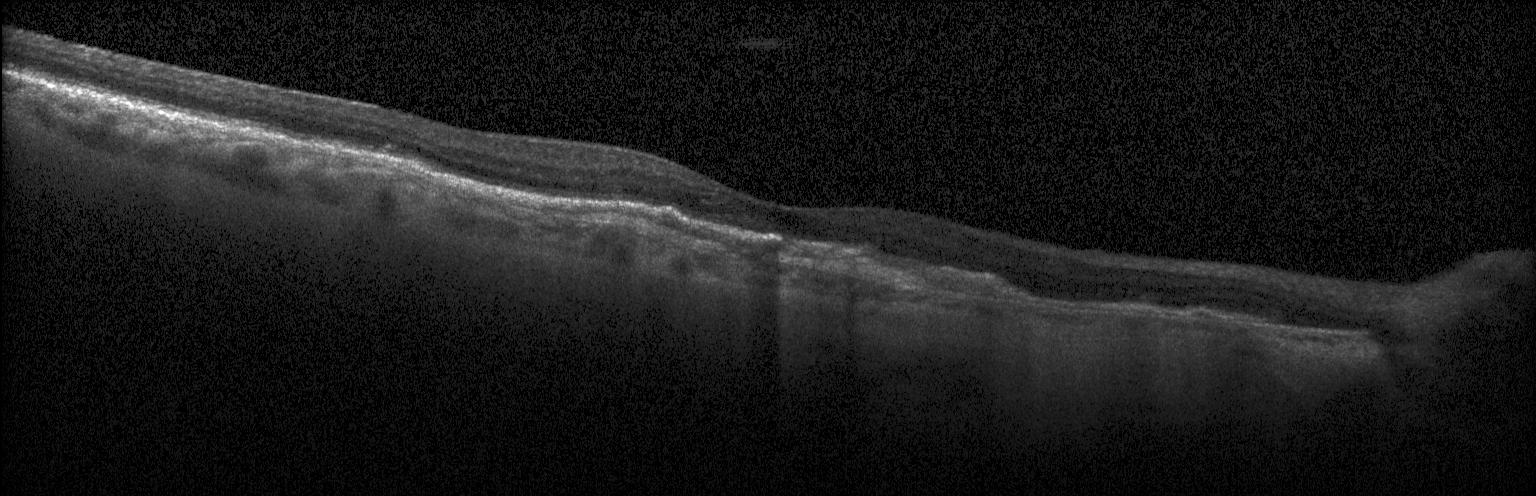 Diagnosis: a choroidal neovascular membrane.